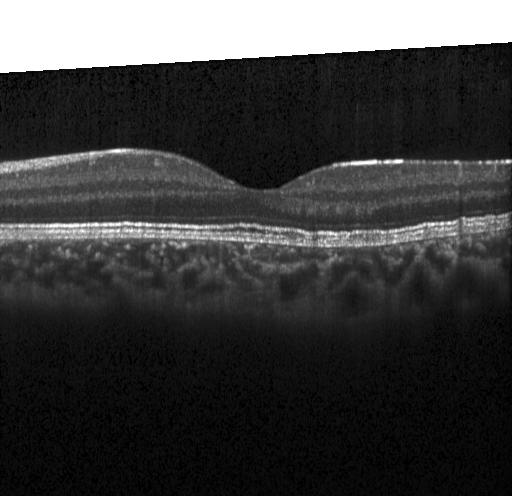
Impression: no CNV, DME, or drusen.